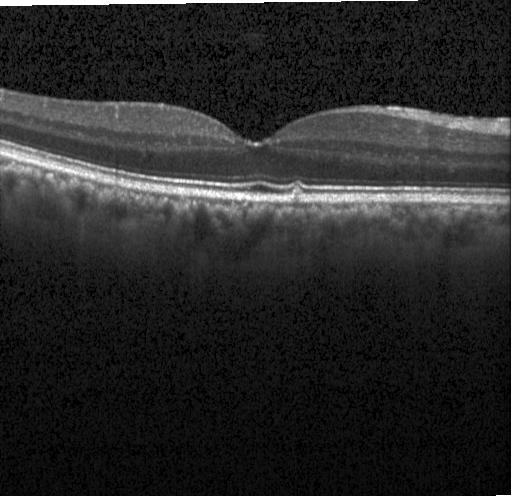 Centered on the fovea. OCT B-scan. Spectral-domain OCT
This B-scan demonstrates sub-RPE drusenoid deposits.